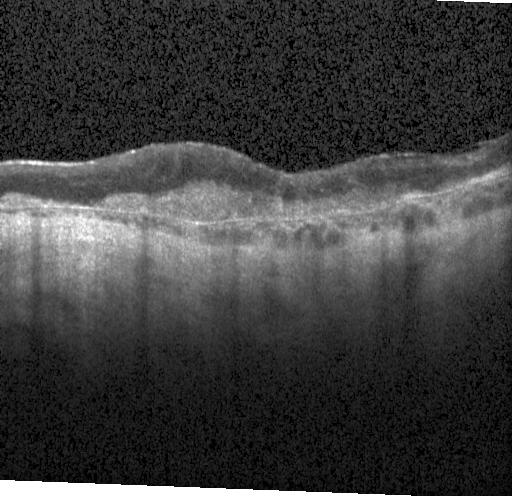
Retinal OCT B-scan. Diagnosis: choroidal neovascularization (CNV).